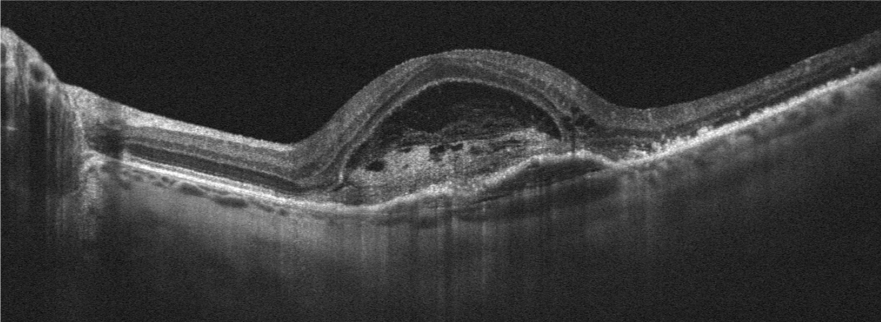
Macular OCT: age-related macular degeneration (AMD).